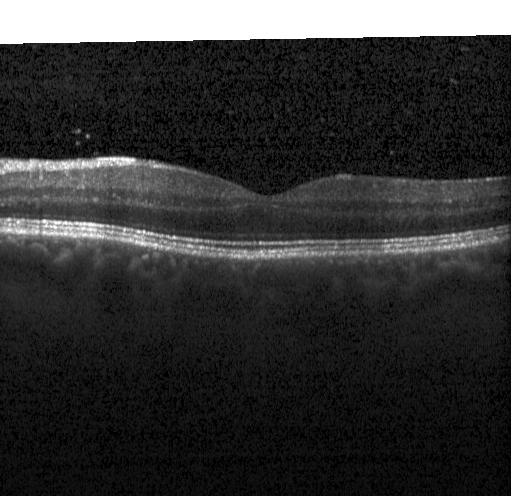

Impression: neither choroidal neovascularization, diabetic macular edema, nor drusen.